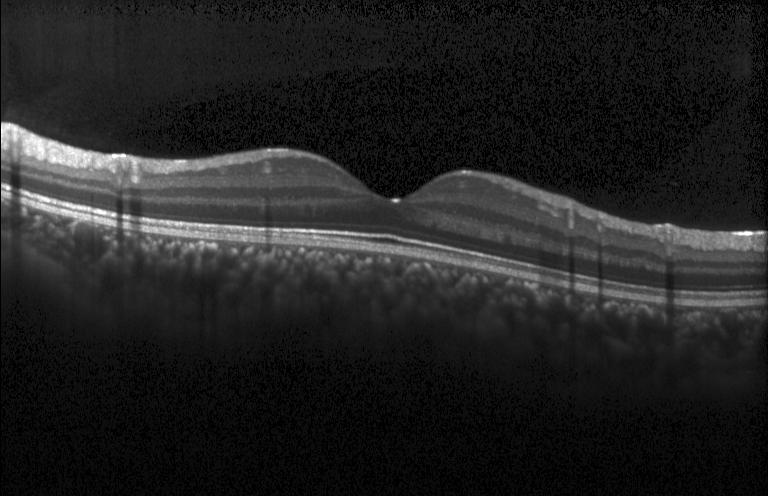 Optical coherence tomography scan; spectral-domain optical coherence tomography; through the macula. Finding: no choroidal neovascularization, diabetic macular edema, or drusen.